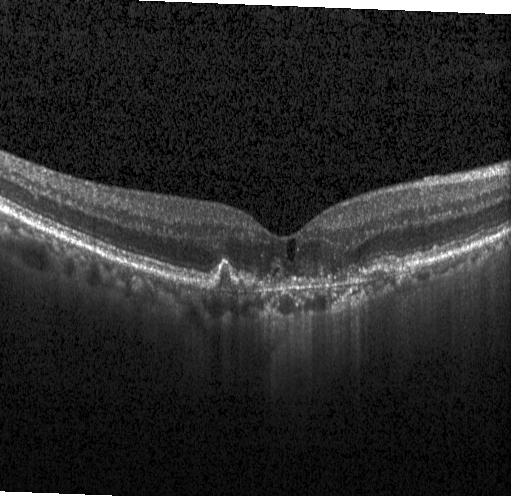

Spectral-domain OCT, fovea-centered, acquired on a Heidelberg Spectralis, retinal OCT B-scan
Diagnosis: CNV.